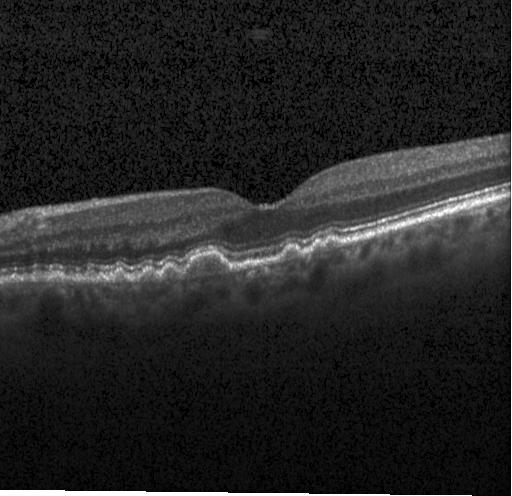 Assessment: multiple drusen.